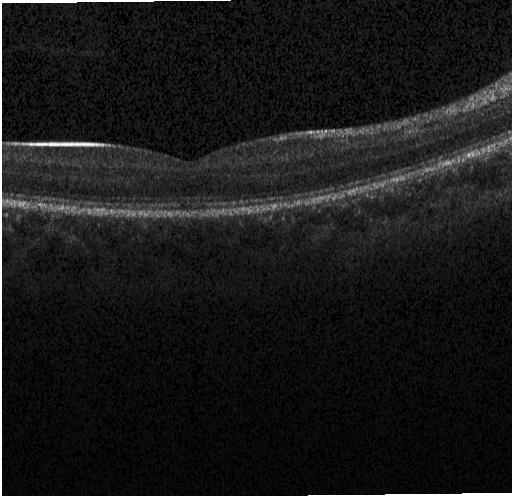
OCT line scan.
Macular OCT: no CNV, no DME, and no drusen.